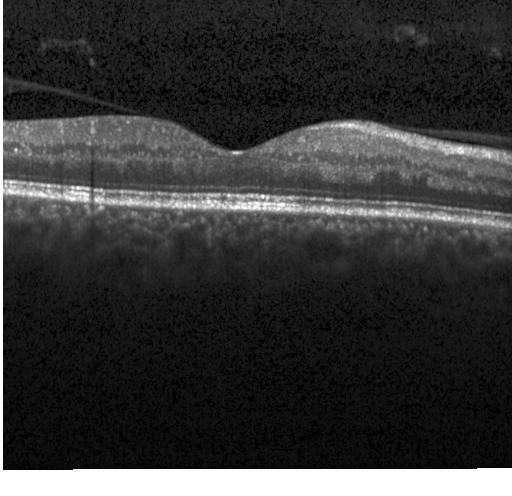
OCT finding: no CNV, no DME, and no drusen.